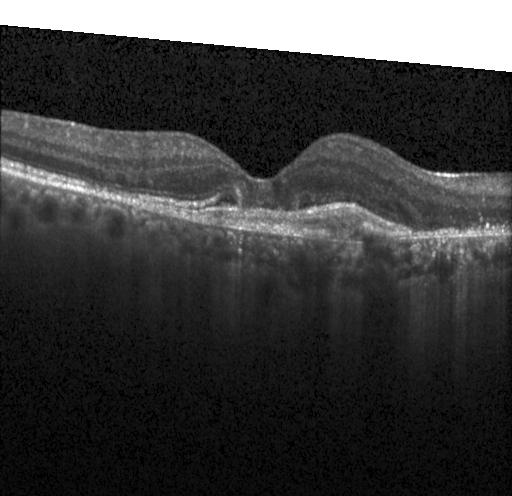 Retinal OCT cross-section showing a choroidal neovascular membrane.